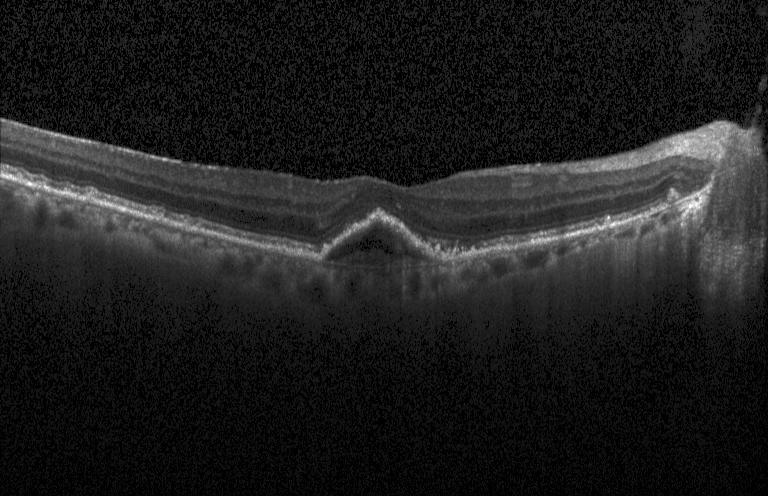 OCT B-scan showing choroidal neovascularization.